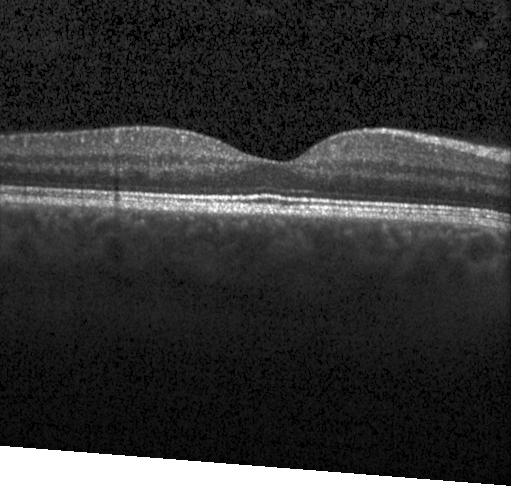
No CNV, no DME, and no drusen.